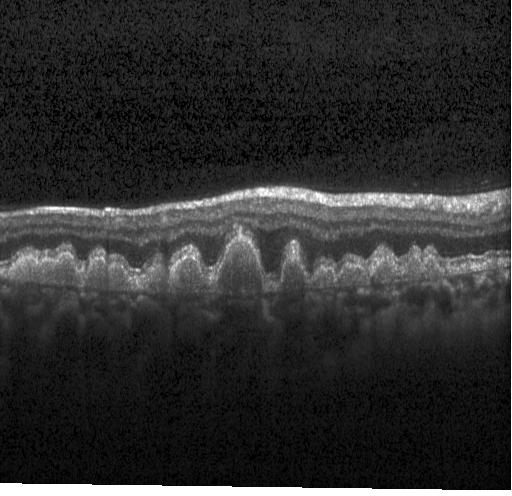 OCT line scan; instrument: Heidelberg Spectralis; spectral-domain OCT; fovea-centered — This B-scan demonstrates multiple drusen.